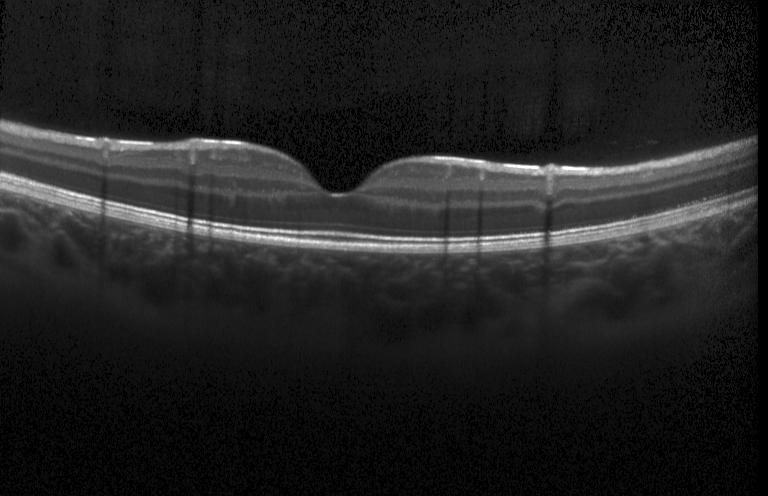

Optical coherence tomography scan, through the macula
Assessment: no choroidal neovascularization, diabetic macular edema, or drusen.